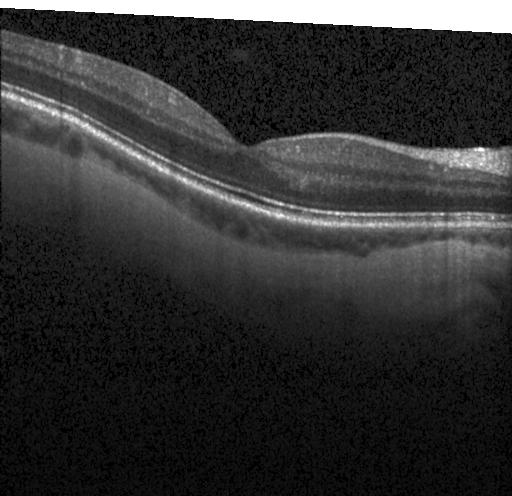 OCT B-scan. Heidelberg Spectralis OCT system. SD-OCT. Fovea-centered.
Macular OCT: neither CNV, DME, nor drusen.